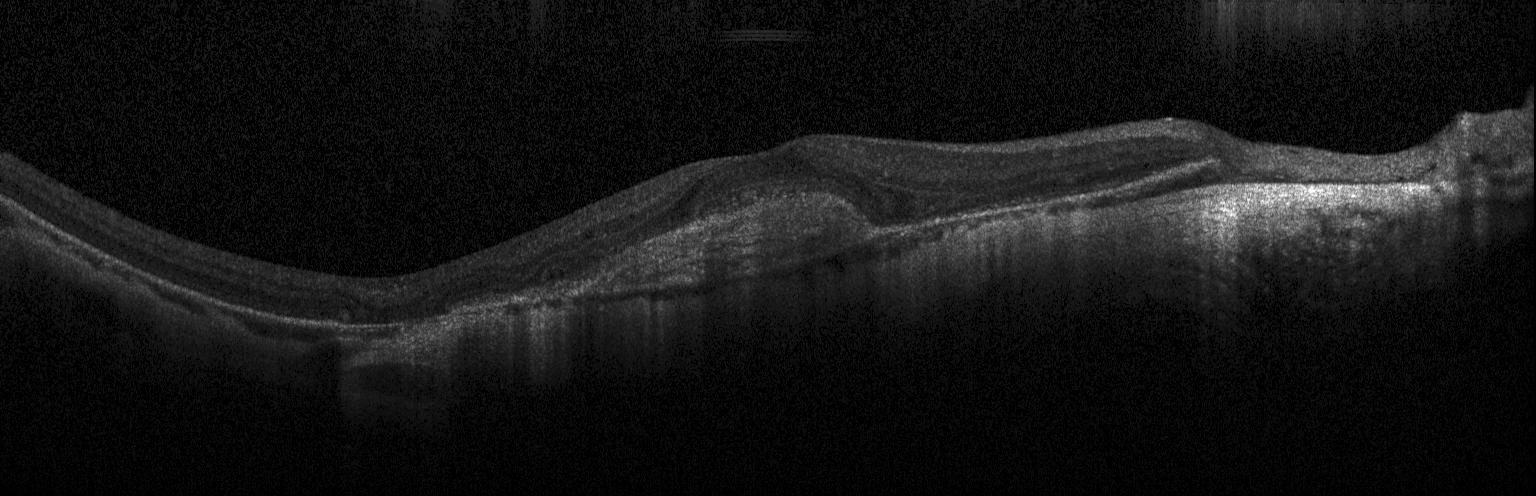 Finding: a choroidal neovascular membrane.